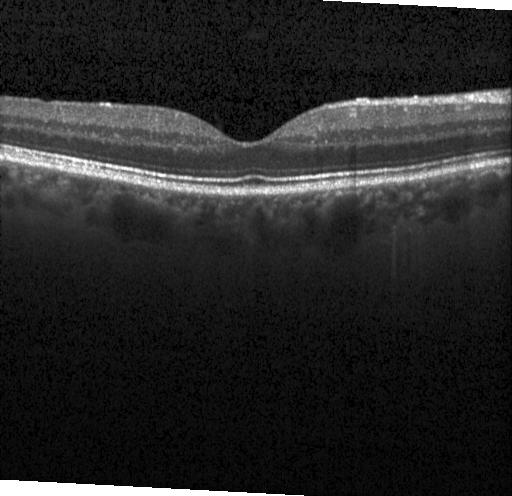
Through the macula · retinal OCT cross-section. Diagnosis: no evidence of CNV, DME, or drusen.